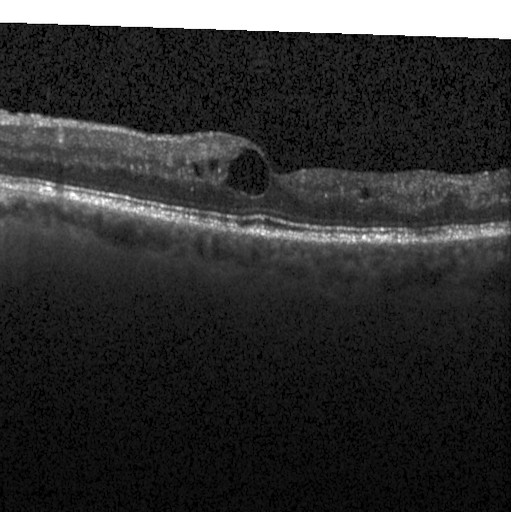

OCT scan showing diabetic macular edema (DME).